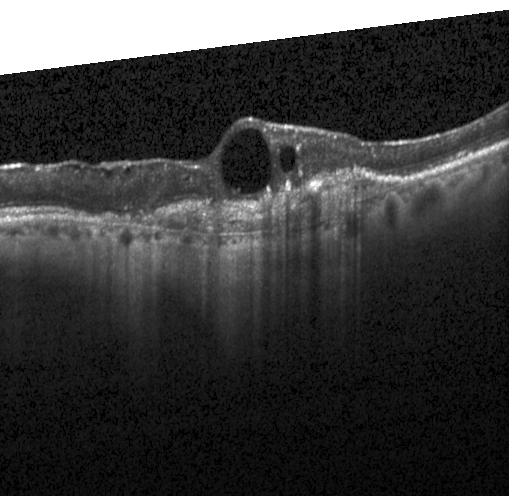
Heidelberg Spectralis, spectral-domain OCT, OCT line scan
A choroidal neovascular membrane.